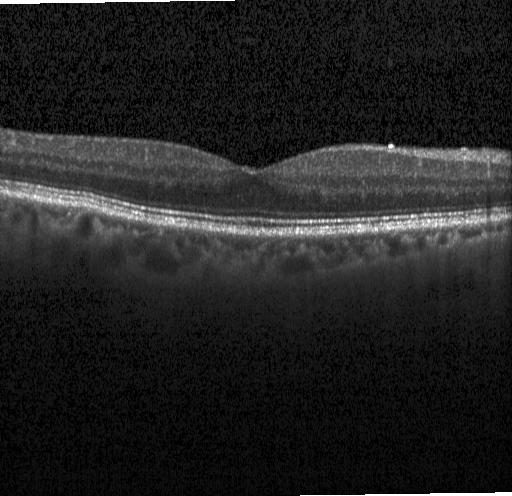 Optical coherence tomography scan.
Impression: no CNV, no DME, and no drusen.